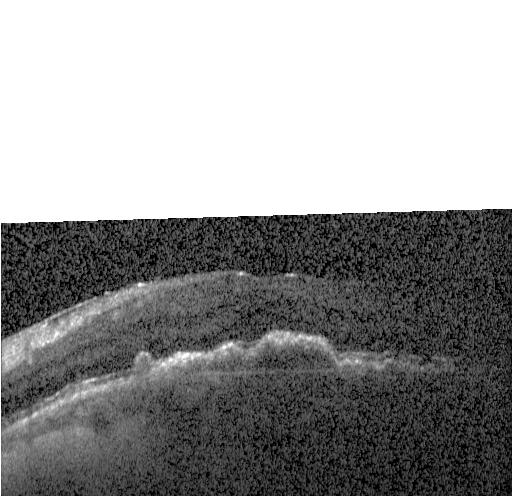

SD-OCT; optical coherence tomography B-scan; horizontal scan through the fovea; Heidelberg Spectralis OCT system
This B-scan demonstrates a choroidal neovascular membrane.